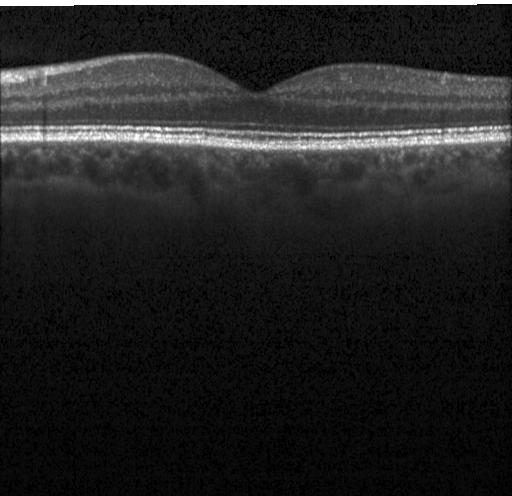 Retinal OCT cross-section · acquired on a Heidelberg Spectralis. OCT finding: no CNV, no DME, and no drusen.